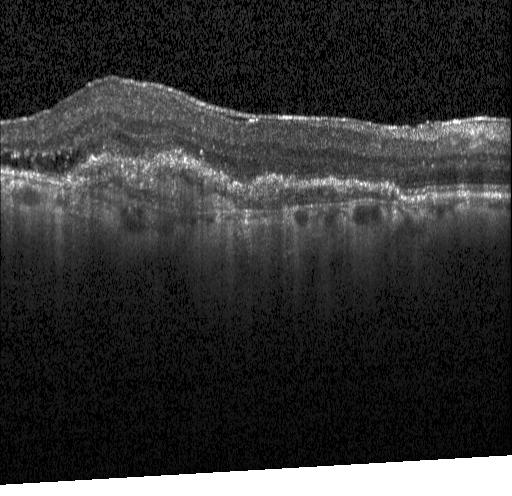
OCT B-scan showing choroidal neovascularization.